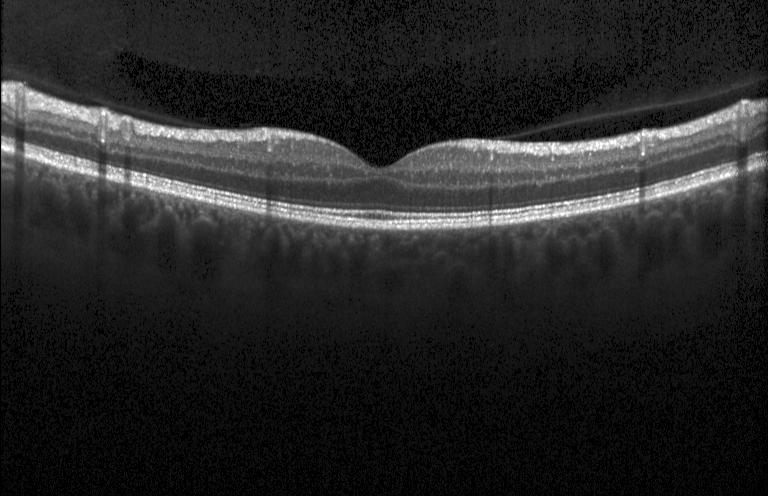

Diagnosis: no choroidal neovascularization, no diabetic macular edema, and no drusen.